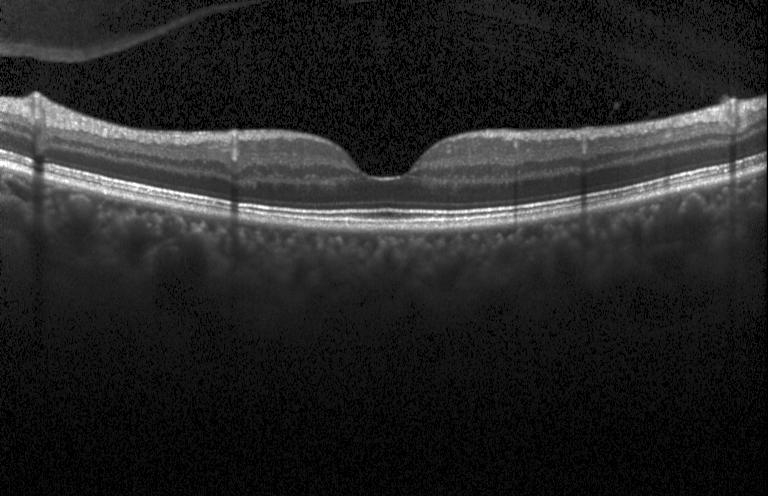

OCT scan showing no choroidal neovascularization, diabetic macular edema, or drusen.